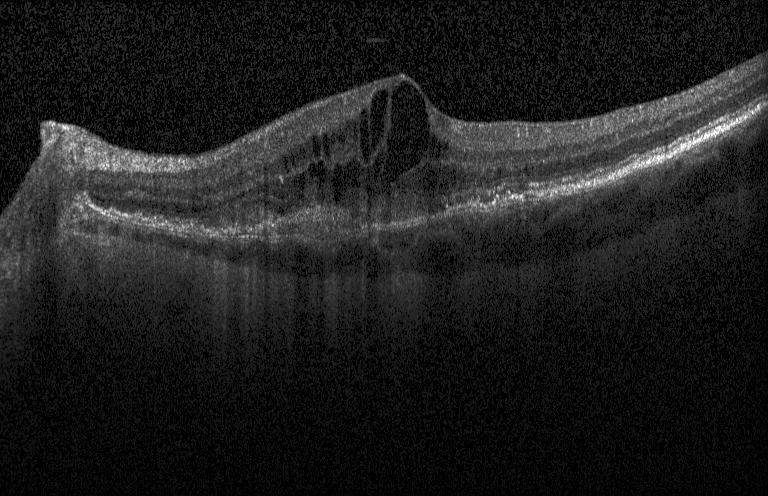

OCT B-scan showing a choroidal neovascular membrane.